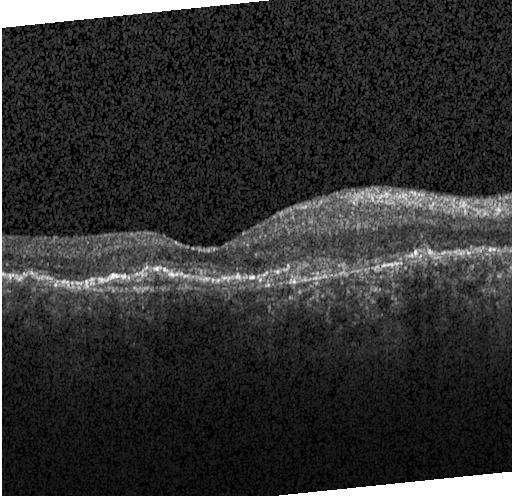 Optical coherence tomography B-scan
Dx: a choroidal neovascular membrane.